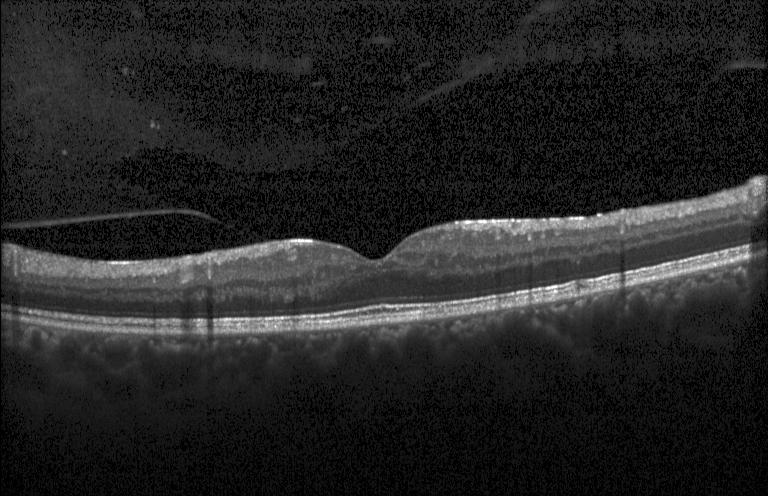

Diagnosis: neither choroidal neovascularization, diabetic macular edema, nor drusen.